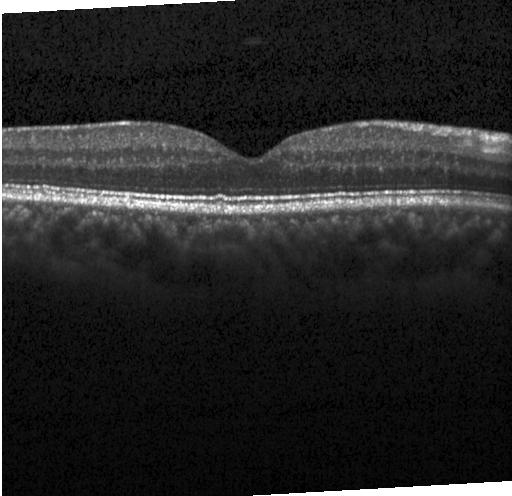
Assessment: no choroidal neovascularization, no diabetic macular edema, and no drusen.